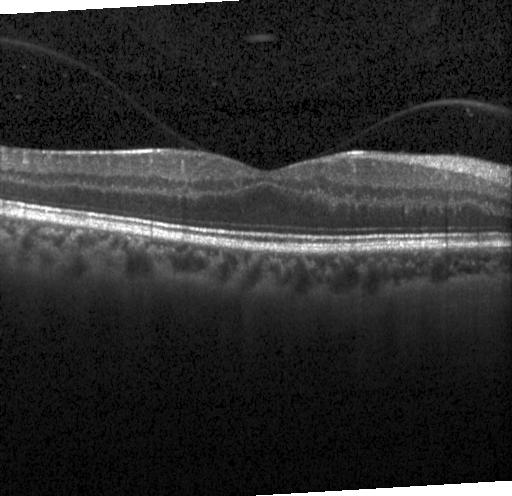
OCT B-scan showing neither choroidal neovascularization, diabetic macular edema, nor drusen.